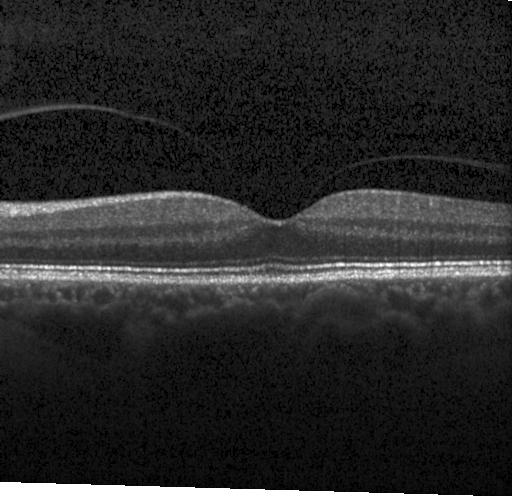

Optical coherence tomography scan
Finding: neither CNV, DME, nor drusen.